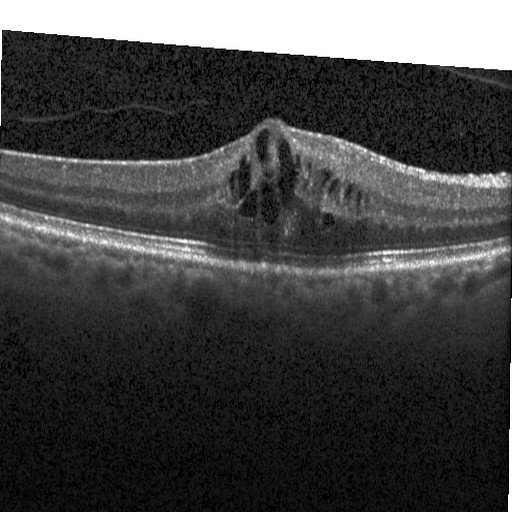 Macular OCT: diabetic macular edema (DME).